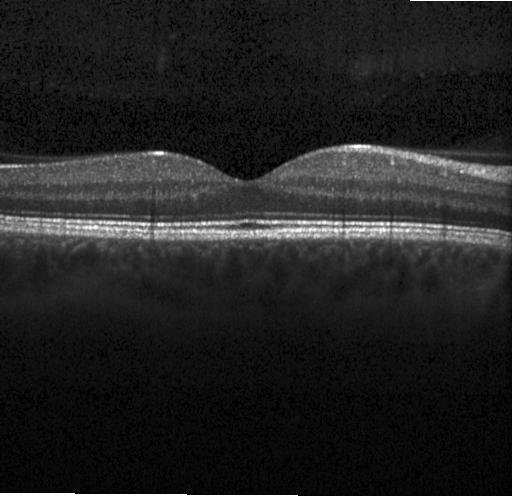 Spectral-domain OCT; retinal OCT cross-section; instrument: Heidelberg Spectralis. This B-scan demonstrates no choroidal neovascularization, no diabetic macular edema, and no drusen.